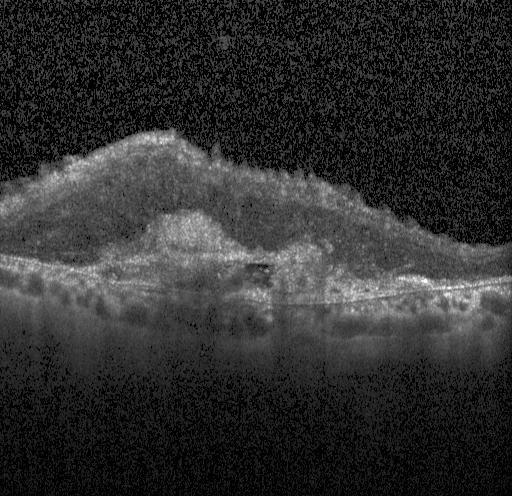

Spectral-domain OCT B-scan: a choroidal neovascular membrane.